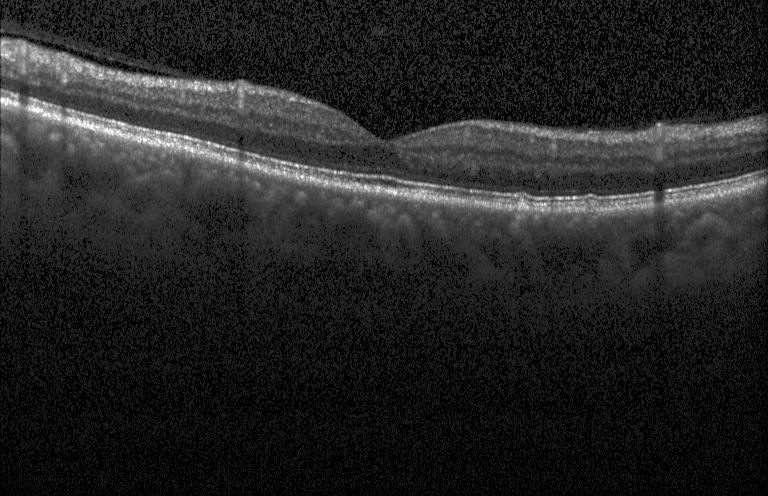

Centered on the fovea, SD-OCT, OCT B-scan, Heidelberg Spectralis OCT system.
Macular OCT: sub-RPE drusenoid deposits.